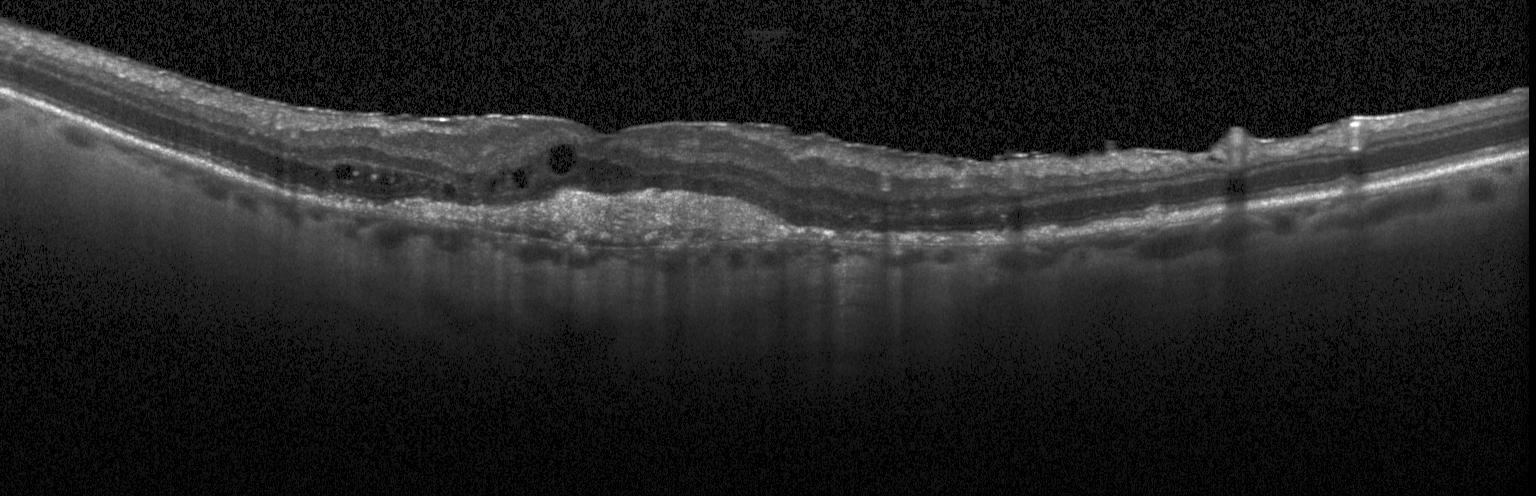 OCT line scan. Diagnosis: choroidal neovascularization.